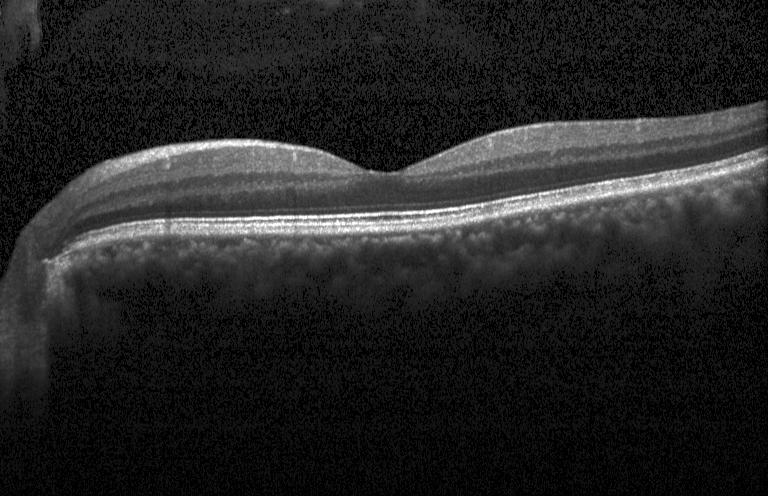 This B-scan demonstrates no choroidal neovascularization, no diabetic macular edema, and no drusen.